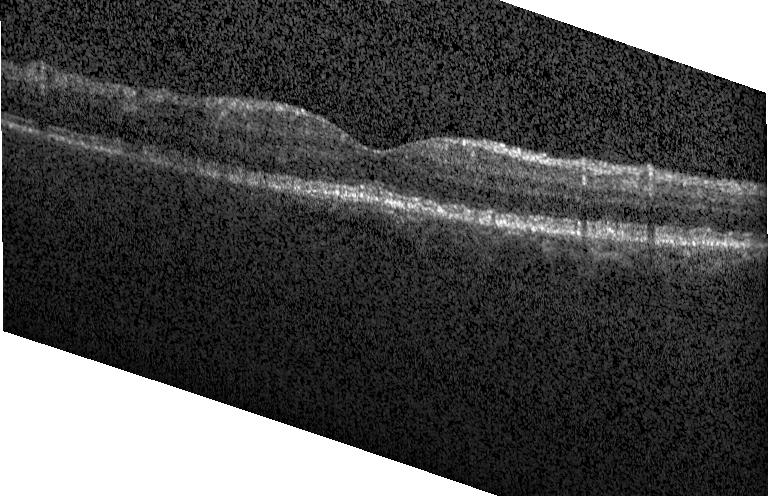
Impression: no evidence of CNV, DME, or drusen.